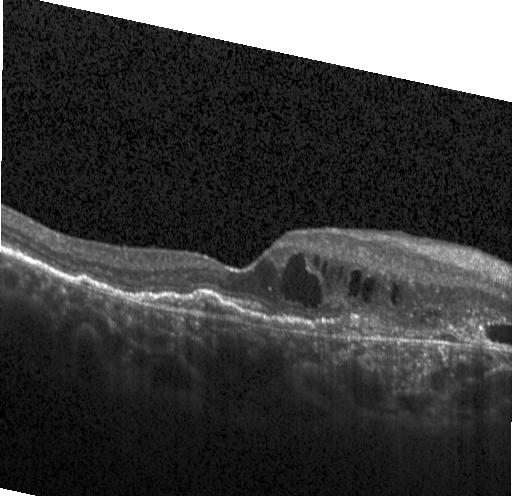

Through the macula; instrument: Heidelberg Spectralis; SD-OCT; OCT B-scan
Macular OCT: a choroidal neovascular membrane.